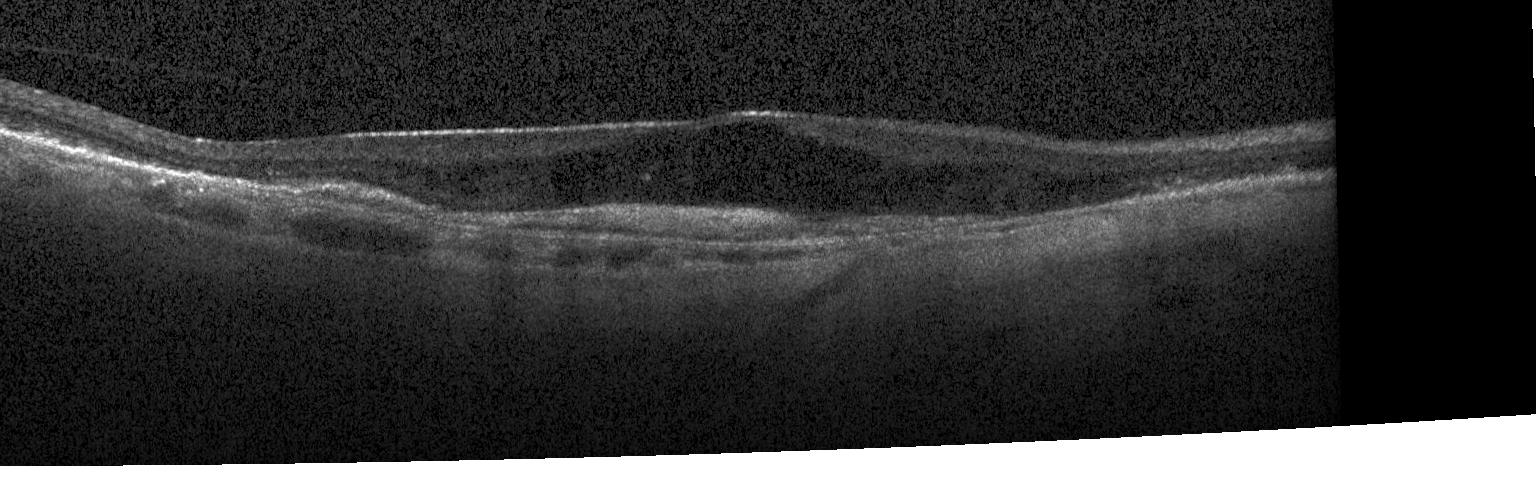

Optical coherence tomography scan
Impression: a choroidal neovascular membrane.